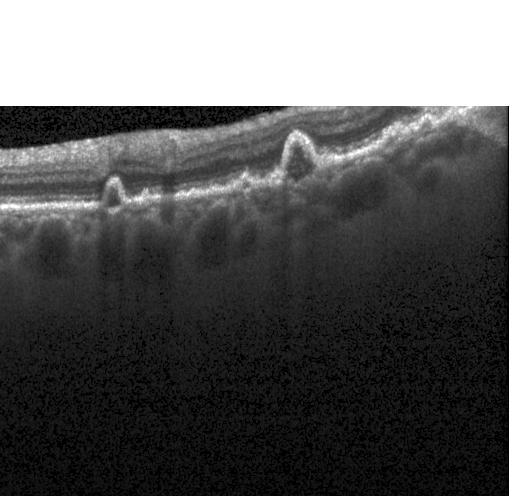

Finding: CNV.